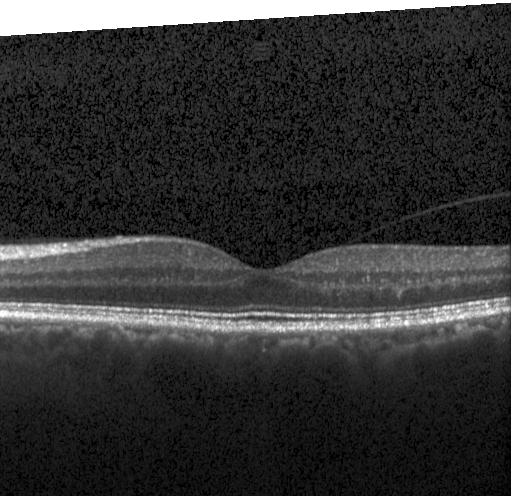
No evidence of CNV, DME, or drusen.